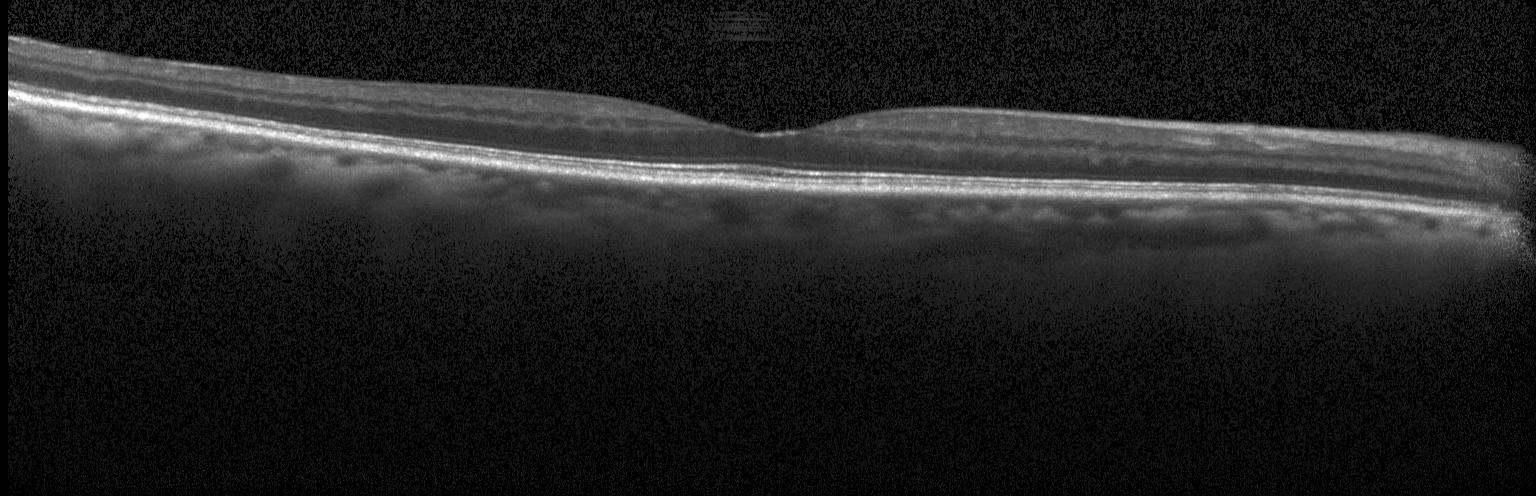
Impression: no choroidal neovascularization, no diabetic macular edema, and no drusen.